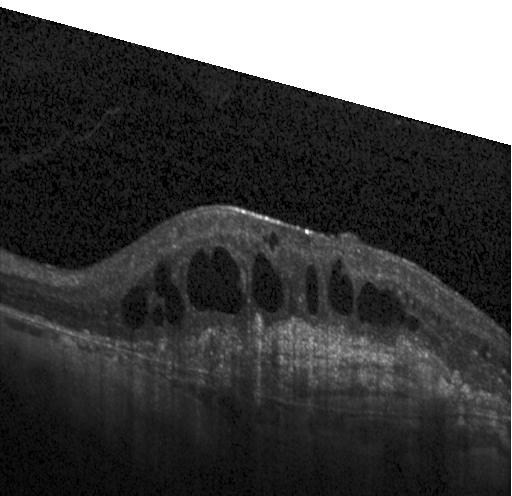

Finding: a choroidal neovascular membrane.